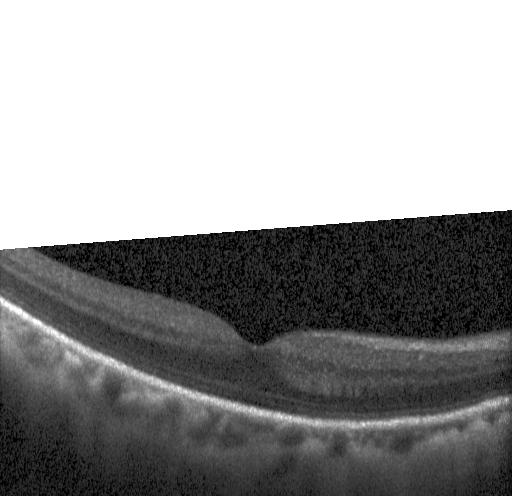

Retinal OCT cross-section
Diagnosis: no choroidal neovascularization, diabetic macular edema, or drusen.